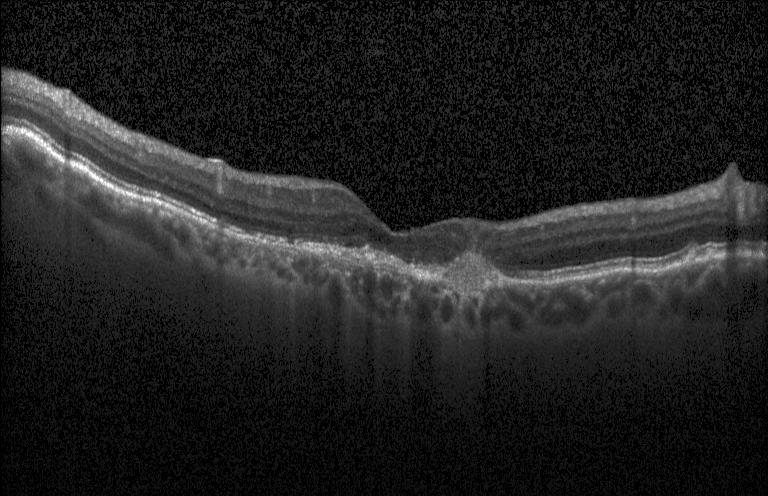 Assessment: a choroidal neovascular membrane.